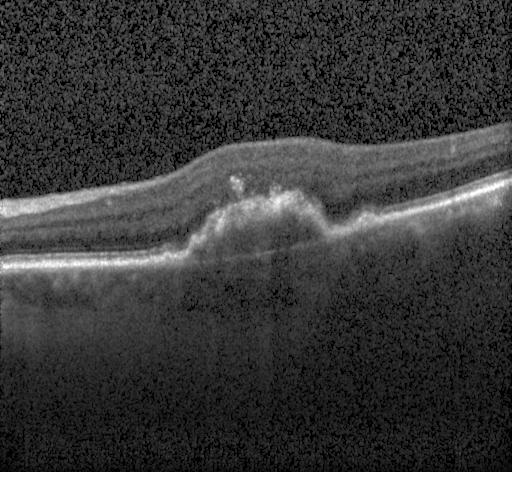

OCT B-scan showing a choroidal neovascular membrane.